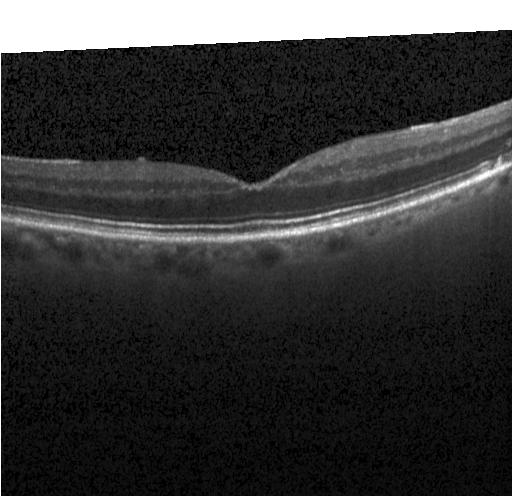 Finding: no CNV, DME, or drusen.